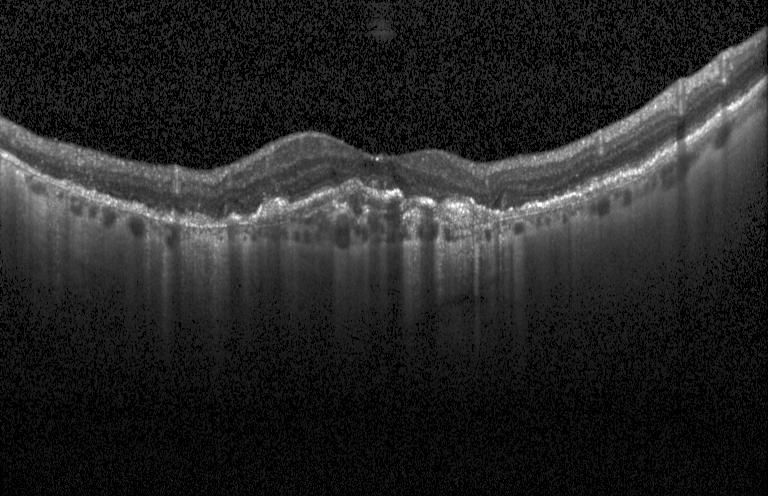

SD-OCT · retinal OCT B-scan. Assessment: a choroidal neovascular membrane.